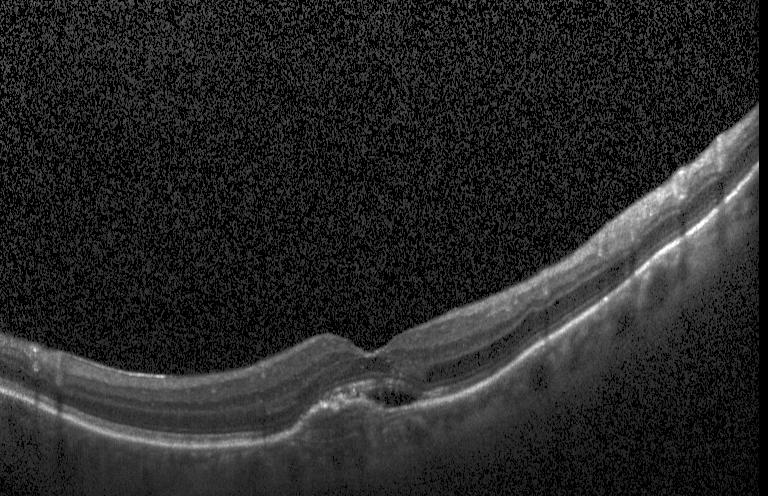
Instrument: Heidelberg Spectralis, macular scan, optical coherence tomography scan
Impression: choroidal neovascularization (CNV).